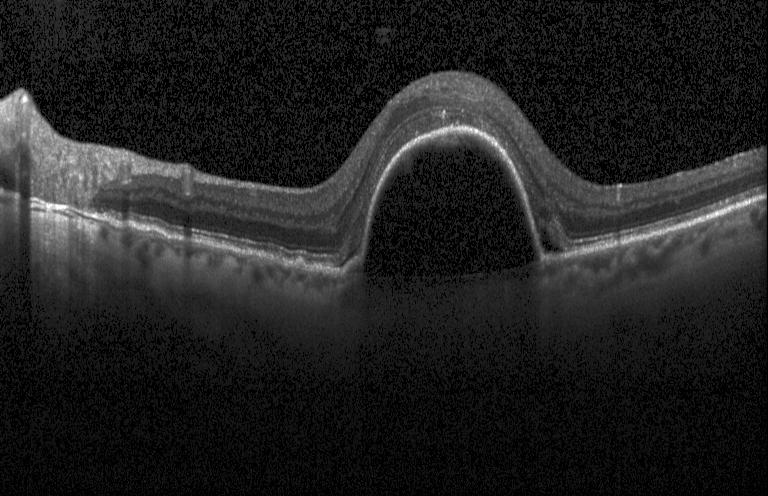

Diagnosis: choroidal neovascularization.